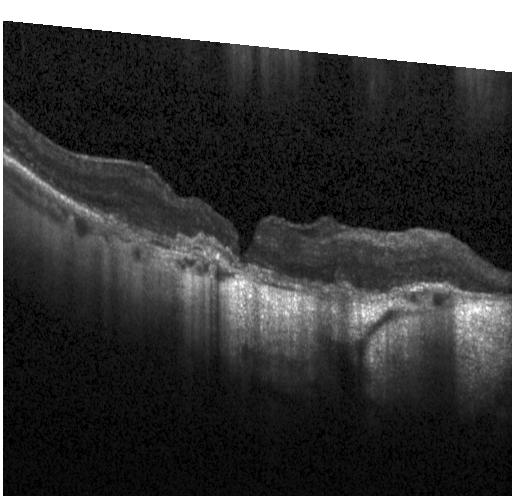
SD-OCT · acquired on a Heidelberg Spectralis · retinal OCT cross-section · centered on the fovea — A choroidal neovascular membrane.